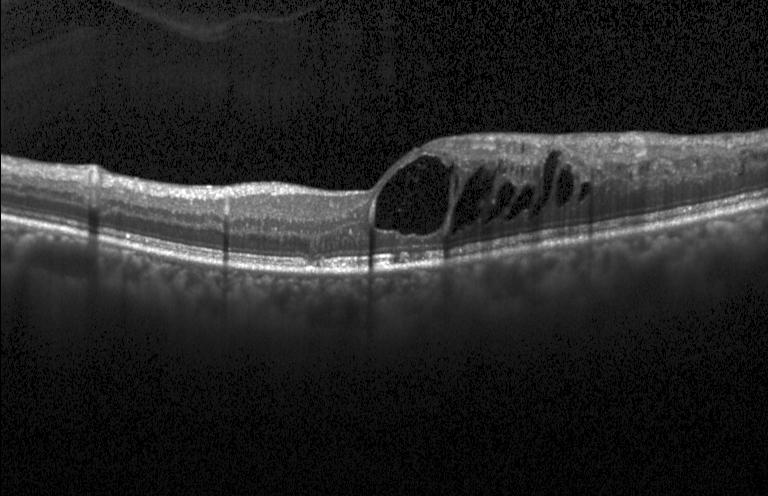 DME.